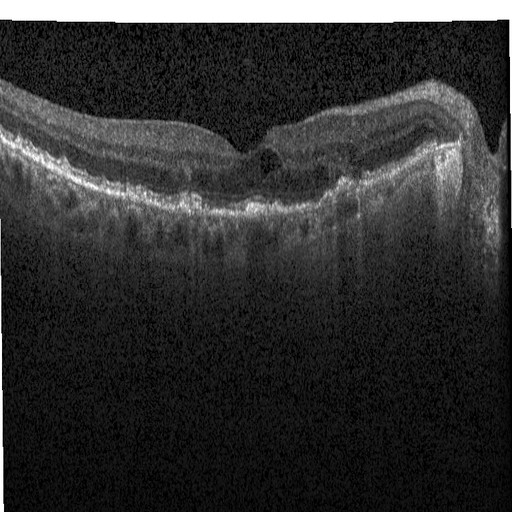
Impression: diabetic macular edema (DME).